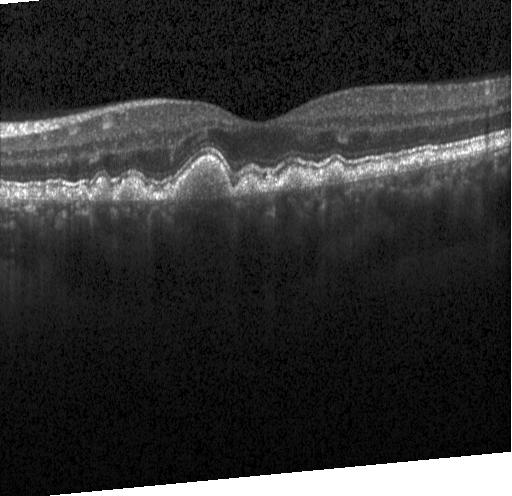
Macular scan; instrument: Heidelberg Spectralis; retinal OCT cross-section; SD-OCT.
Finding: multiple drusen.